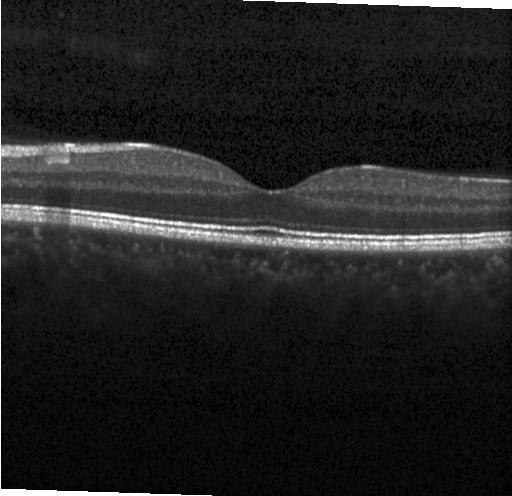

Finding: neither choroidal neovascularization, diabetic macular edema, nor drusen.